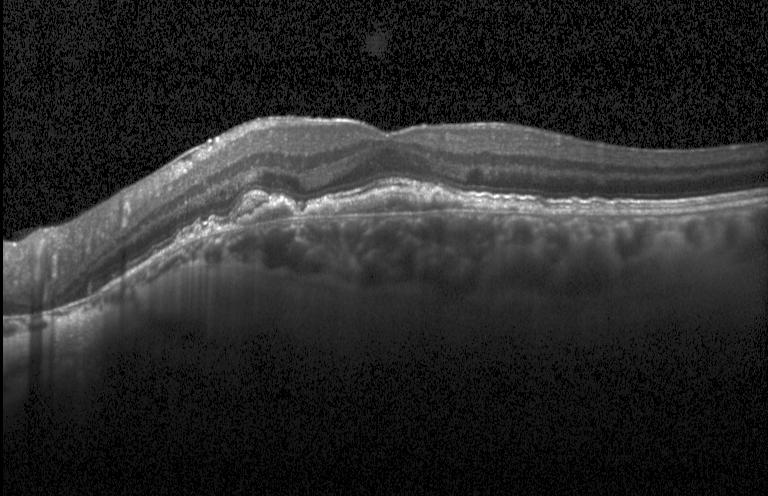
The scan shows a choroidal neovascular membrane.